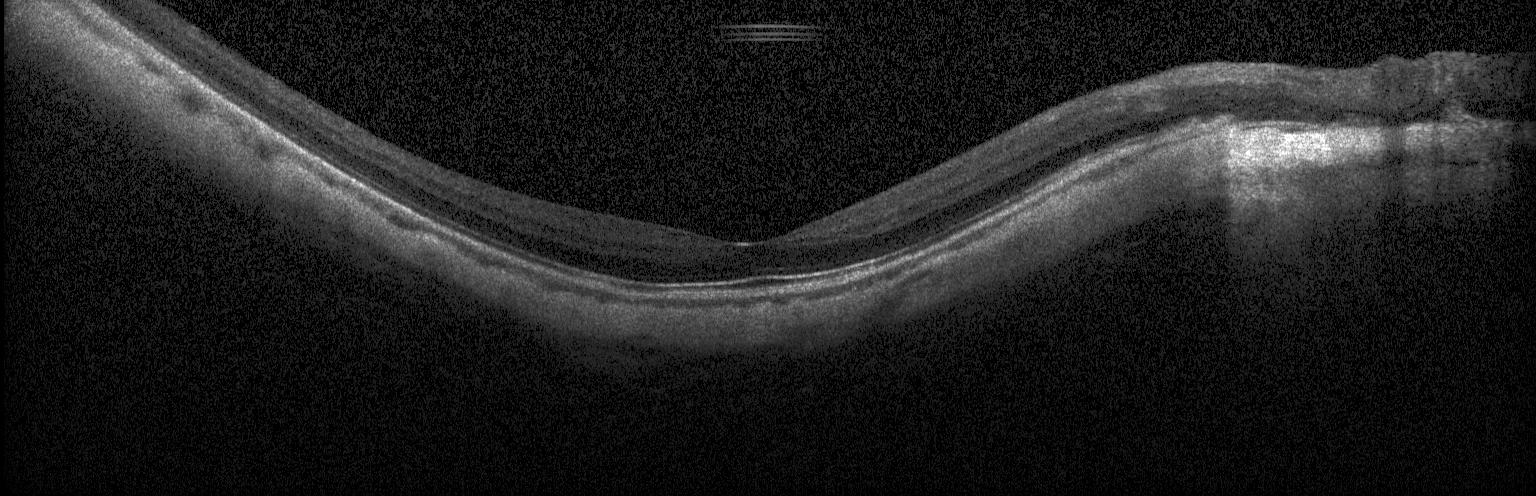 Impression: neither CNV, DME, nor drusen.